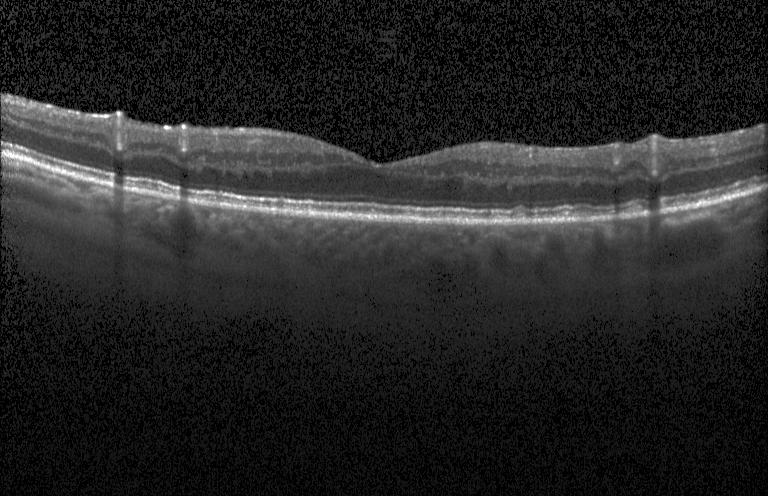 Optical coherence tomography scan. Spectral-domain OCT. Heidelberg Spectralis OCT system. Fovea-centered — Impression: drusen.